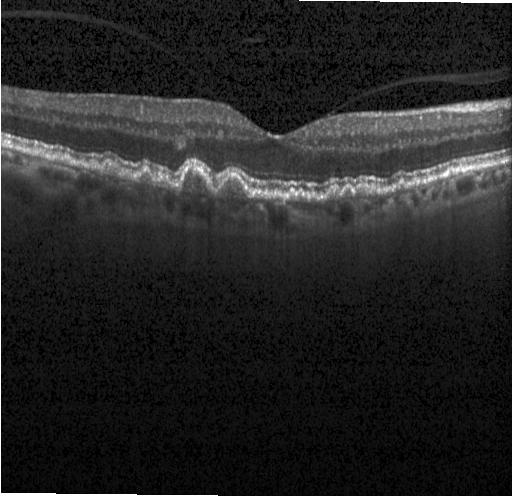

This B-scan demonstrates sub-RPE drusenoid deposits.